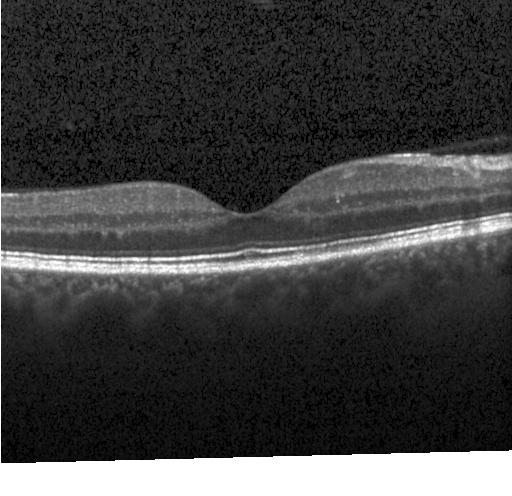

Spectral-domain optical coherence tomography; acquired on a Heidelberg Spectralis; OCT line scan; centered on the fovea. The scan shows no CNV, DME, or drusen.